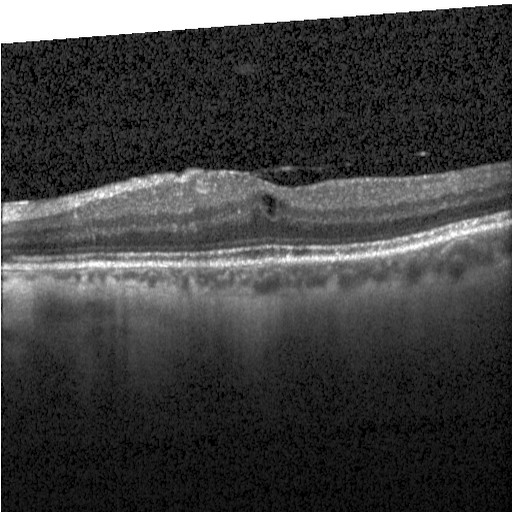 Through the macula · OCT B-scan · SD-OCT.
Finding: diabetic macular edema.